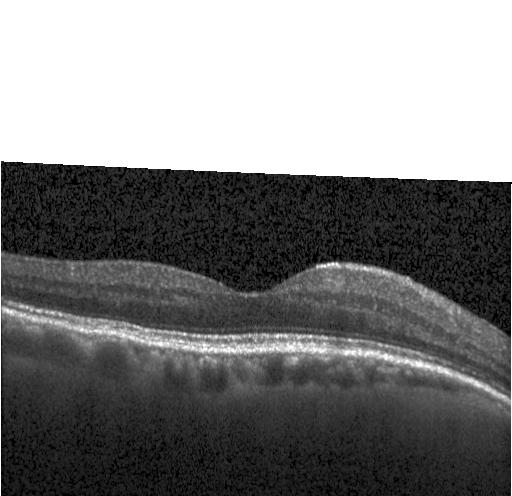
Horizontal scan through the fovea; OCT line scan; SD-OCT; Heidelberg Spectralis — Diagnosis: neither CNV, DME, nor drusen.